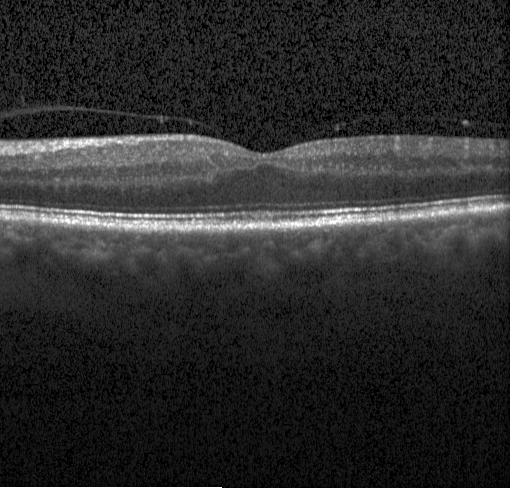
Finding: no choroidal neovascularization, no diabetic macular edema, and no drusen.